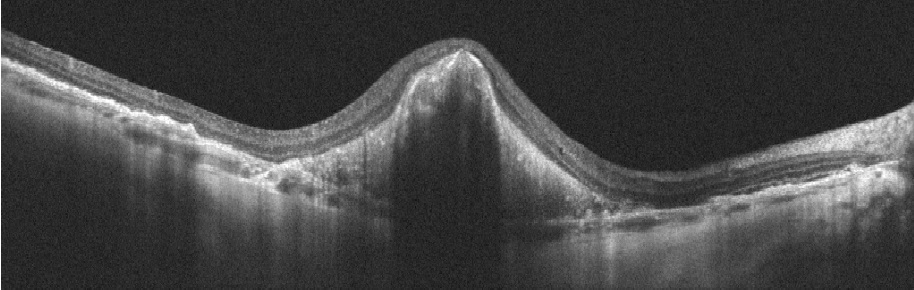

Assessment: age-related macular degeneration.